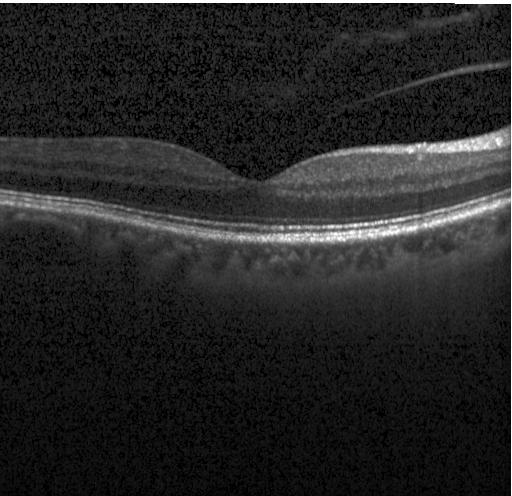
The scan shows no evidence of choroidal neovascularization, diabetic macular edema, or drusen.